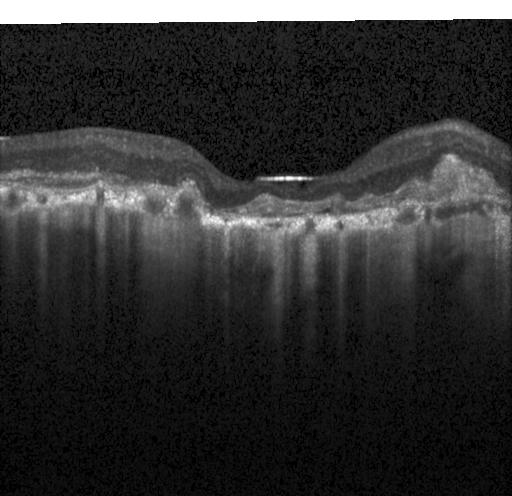 Heidelberg Spectralis. OCT line scan. SD-OCT. Fovea-centered
This B-scan demonstrates CNV.